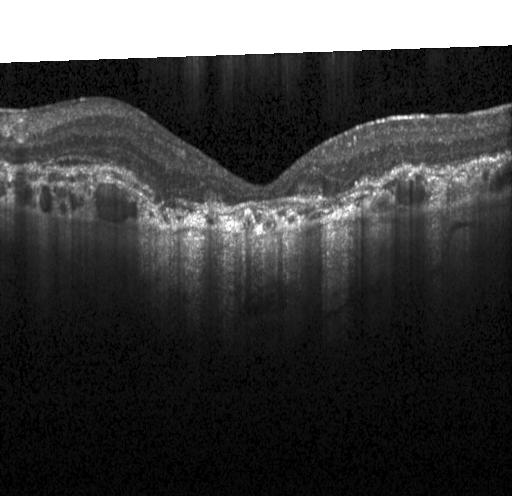

Spectral-domain optical coherence tomography. OCT line scan. Diagnosis: choroidal neovascularization.